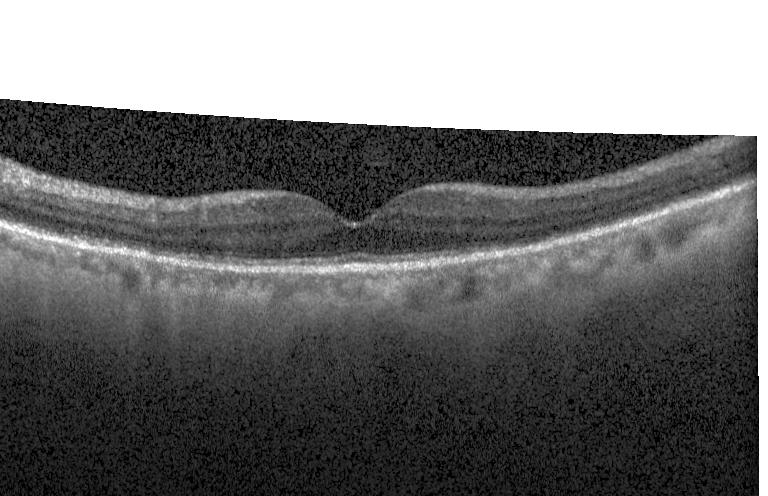
Instrument: Heidelberg Spectralis. OCT B-scan. SD-OCT. Macular scan
This B-scan demonstrates no evidence of CNV, DME, or drusen.